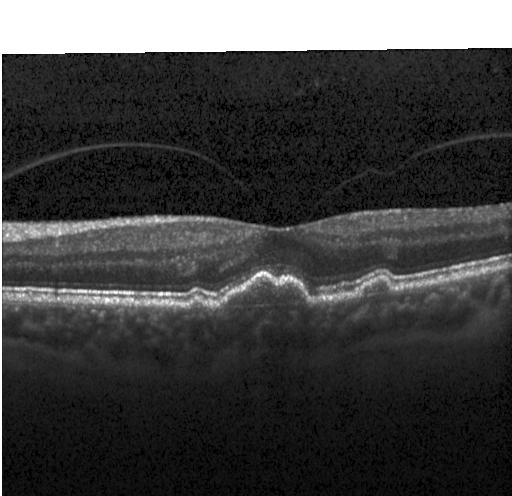

Acquired on a Heidelberg Spectralis. Retinal OCT cross-section. Spectral-domain optical coherence tomography. Macular scan — Sub-RPE drusenoid deposits.